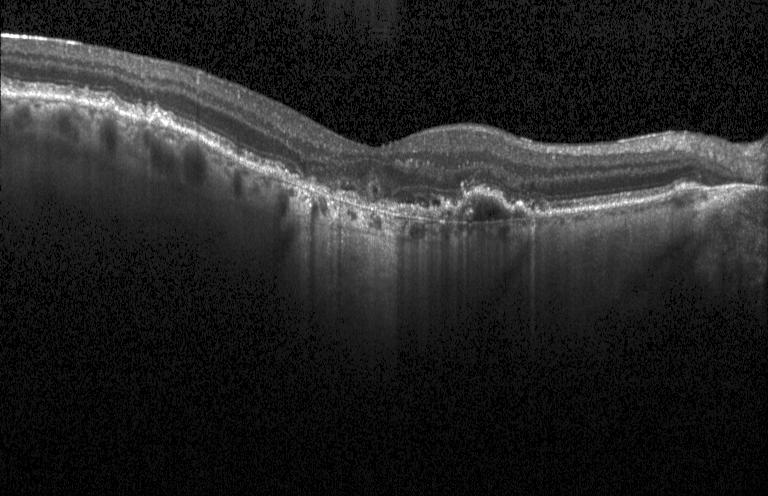

OCT finding: a choroidal neovascular membrane.